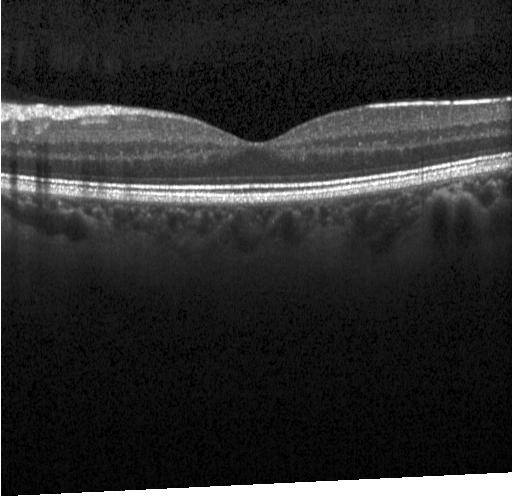 Spectral-domain optical coherence tomography. Retinal OCT cross-section.
Macular OCT: no choroidal neovascularization, diabetic macular edema, or drusen.